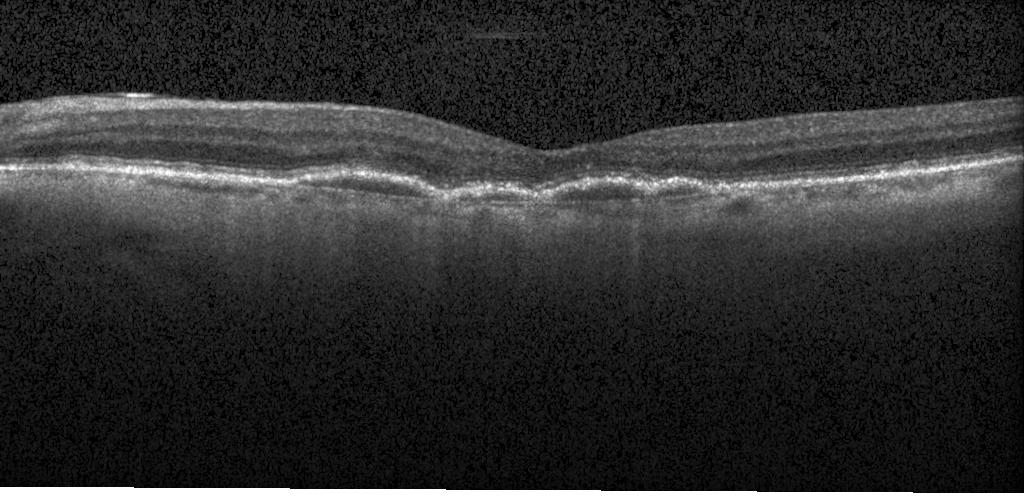
Macular scan · retinal OCT B-scan. CNV.